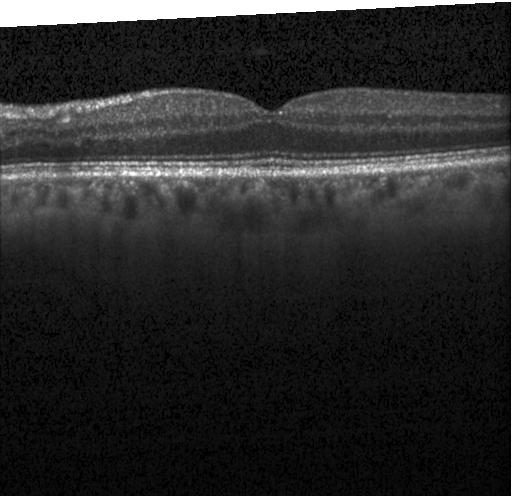 Instrument: Heidelberg Spectralis, spectral-domain OCT, OCT line scan, macular scan. OCT finding: no choroidal neovascularization, diabetic macular edema, or drusen.